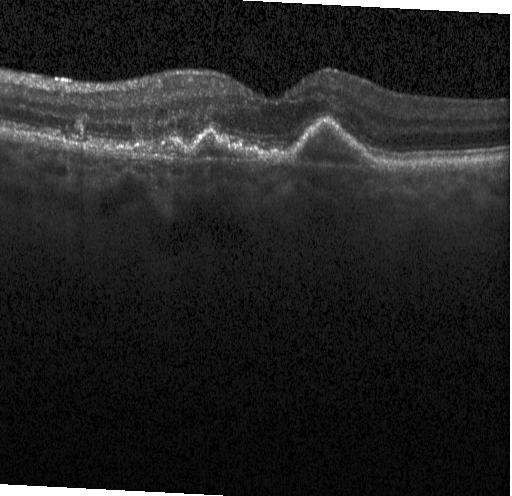

Finding: a choroidal neovascular membrane.